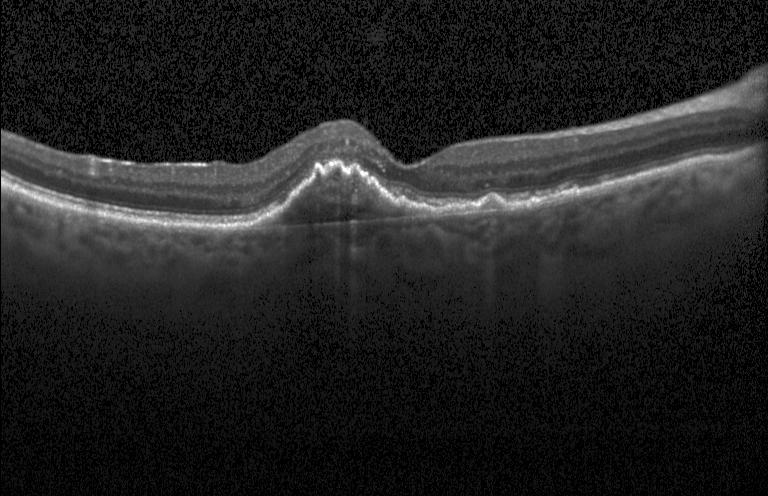
Finding: a choroidal neovascular membrane.